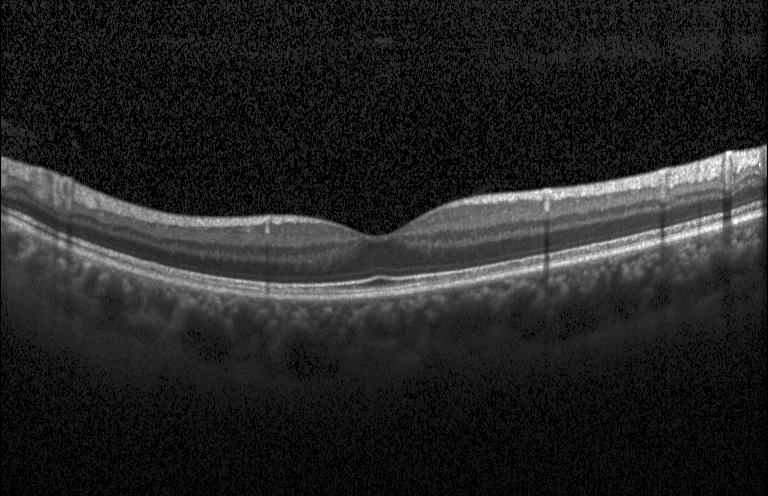
This B-scan demonstrates no choroidal neovascularization, diabetic macular edema, or drusen.